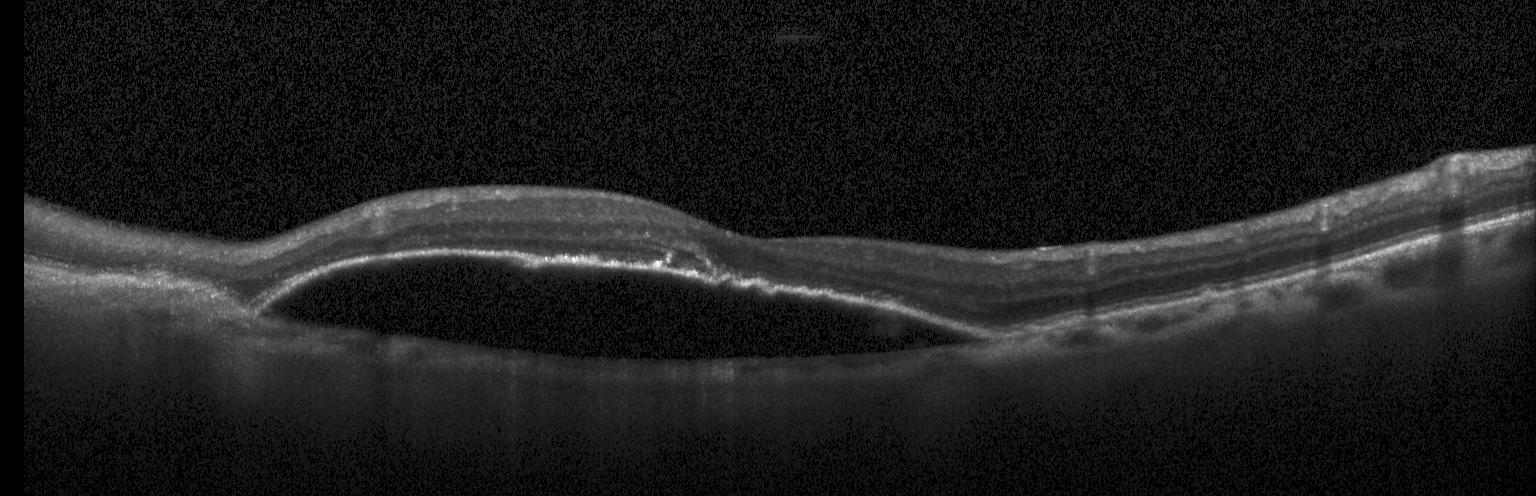 Macular OCT: a choroidal neovascular membrane.